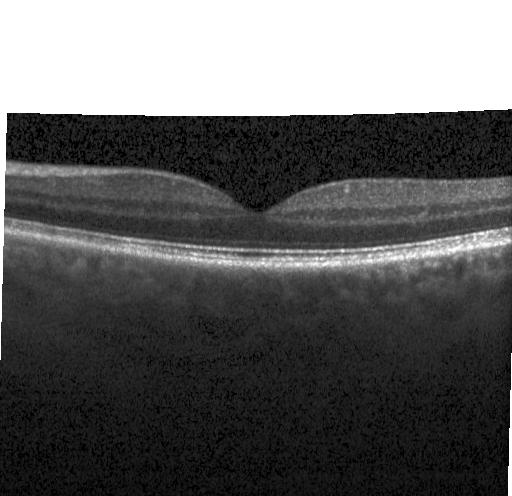

Finding: no choroidal neovascularization, no diabetic macular edema, and no drusen.